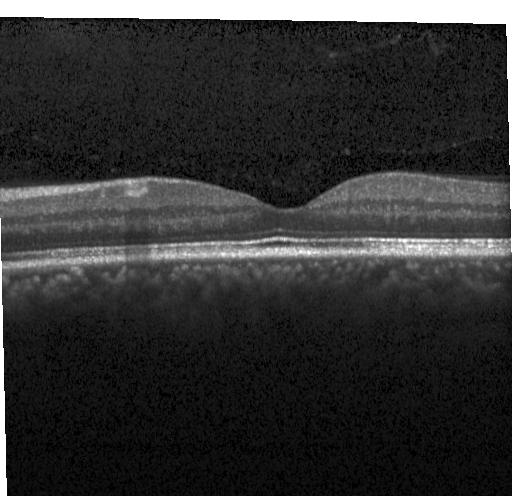

Optical coherence tomography scan
OCT finding: no CNV, no DME, and no drusen.